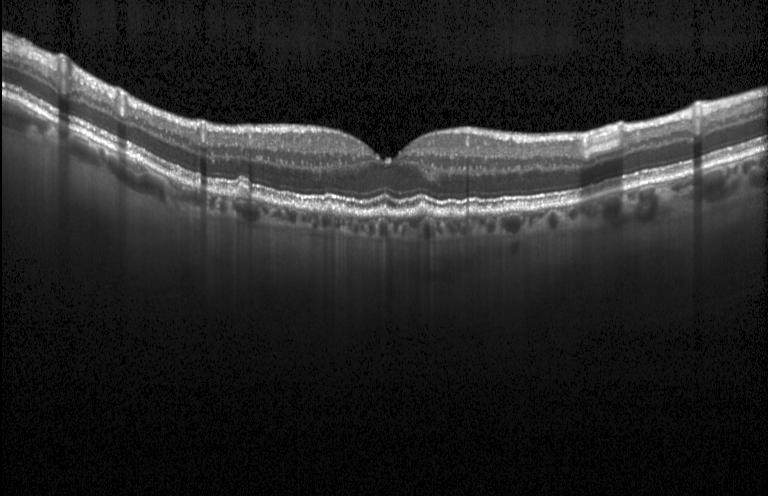 Optical coherence tomography B-scan · acquired on a Heidelberg Spectralis · macular scan · spectral-domain optical coherence tomography.
Finding: sub-RPE drusenoid deposits.